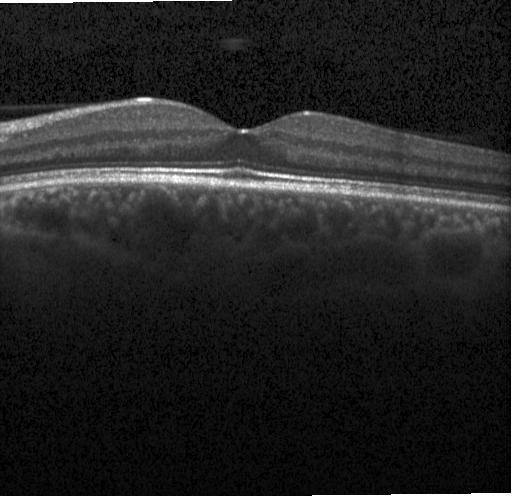 Macular scan, Heidelberg Spectralis, optical coherence tomography scan.
Assessment: no choroidal neovascularization, diabetic macular edema, or drusen.